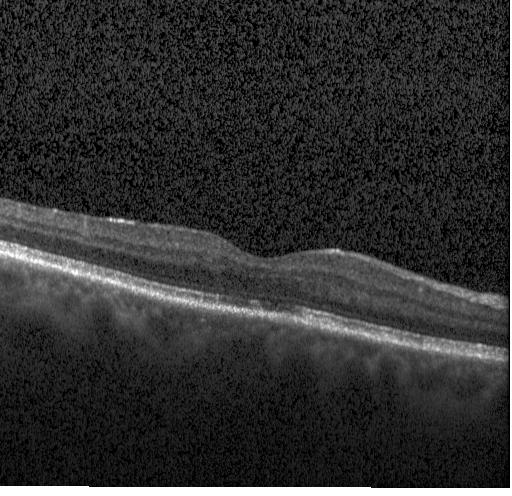

Assessment: no choroidal neovascularization, no diabetic macular edema, and no drusen.